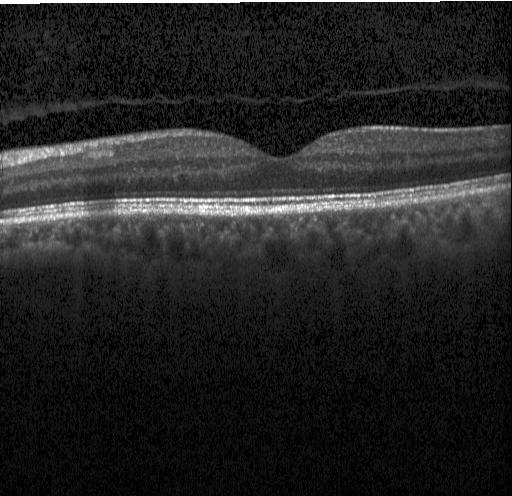 Optical coherence tomography B-scan · Heidelberg Spectralis OCT system · spectral-domain optical coherence tomography. Diagnosis: no choroidal neovascularization, no diabetic macular edema, and no drusen.